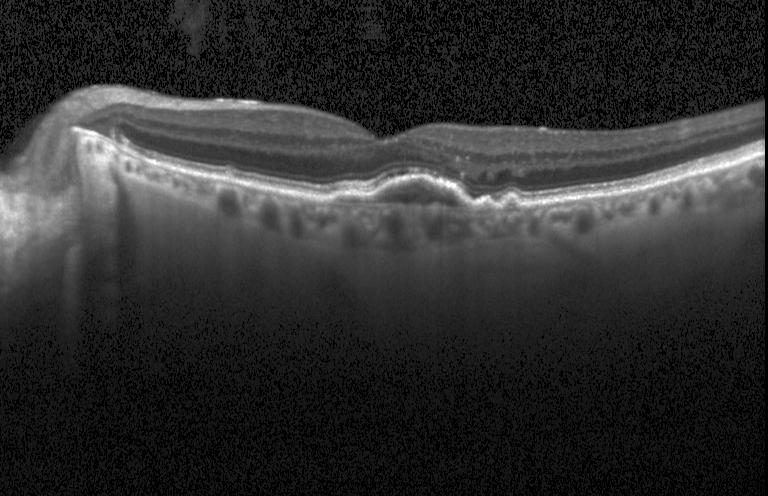

This B-scan demonstrates choroidal neovascularization (CNV).